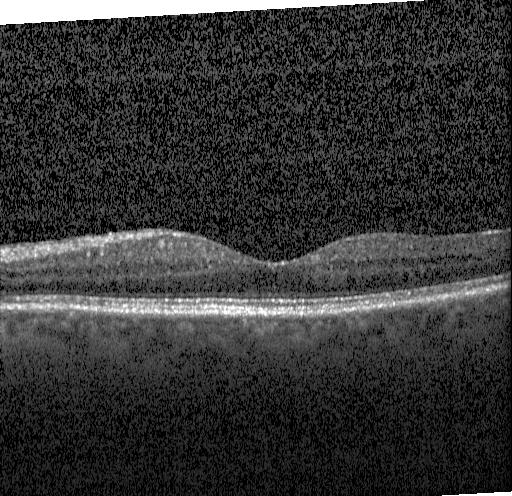
Spectral-domain OCT, optical coherence tomography scan.
This B-scan demonstrates no choroidal neovascularization, no diabetic macular edema, and no drusen.